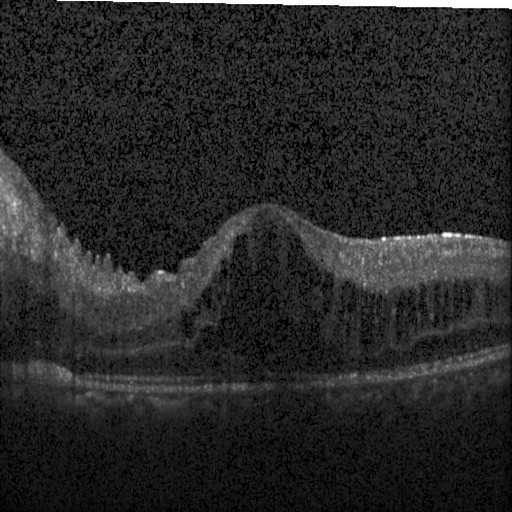 Diagnosis: diabetic macular edema (DME).